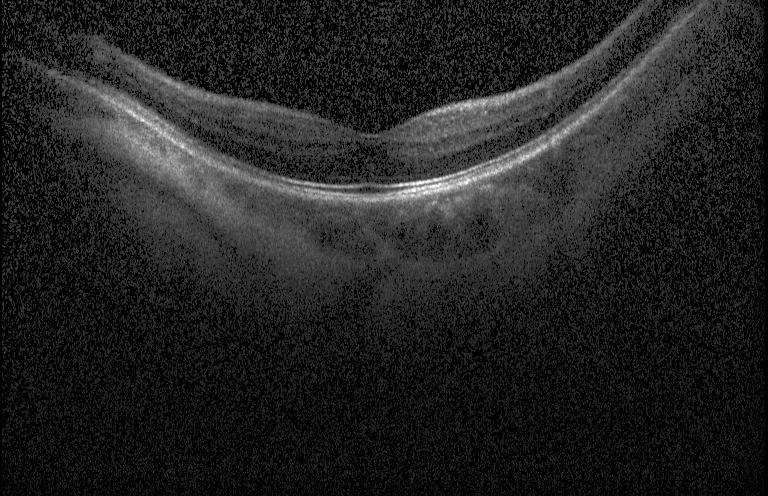 Heidelberg Spectralis. Optical coherence tomography B-scan — This B-scan demonstrates no choroidal neovascularization, diabetic macular edema, or drusen.